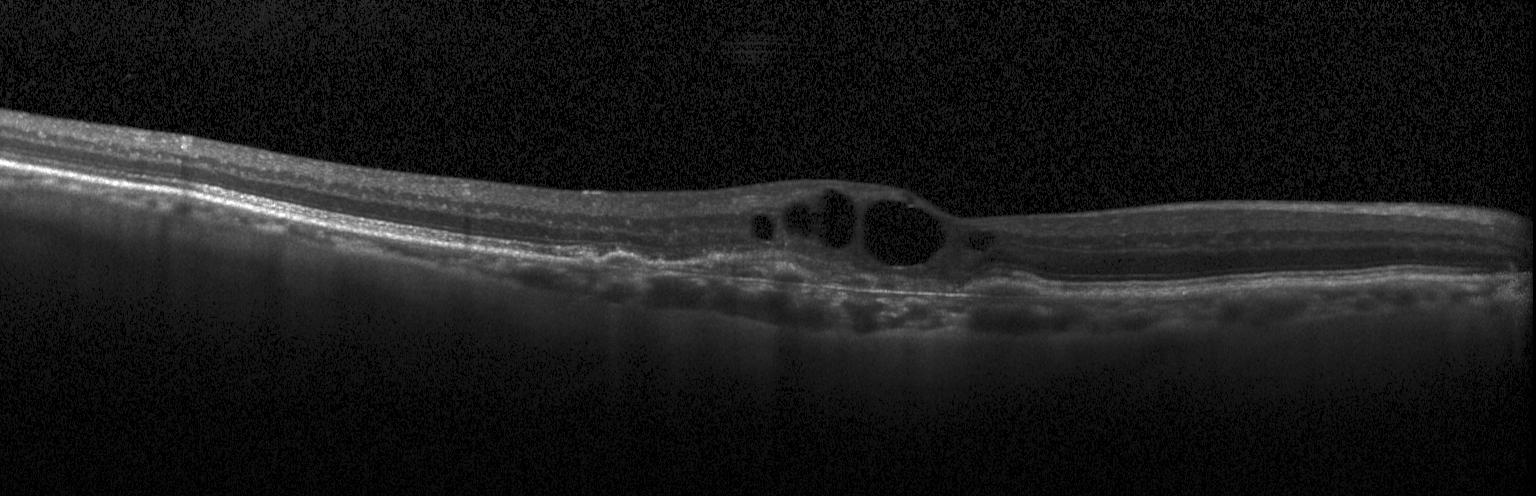 Heidelberg Spectralis OCT system; OCT B-scan; SD-OCT. Finding: a choroidal neovascular membrane.